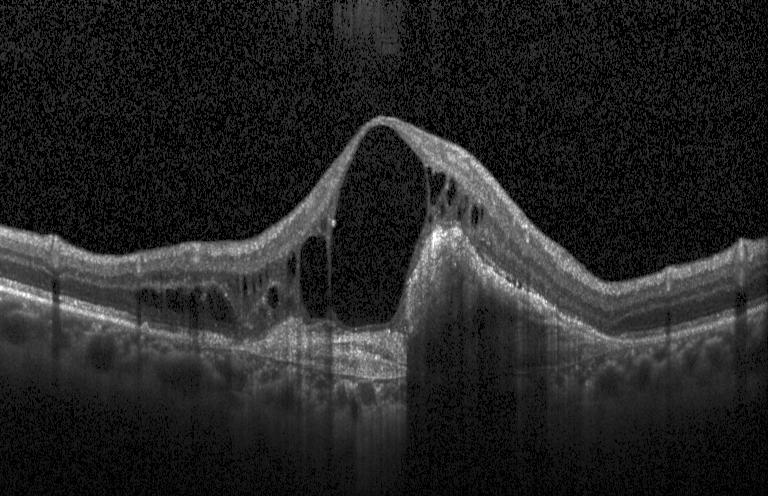 Heidelberg Spectralis OCT system · macular scan · optical coherence tomography B-scan · SD-OCT — Impression: a choroidal neovascular membrane.